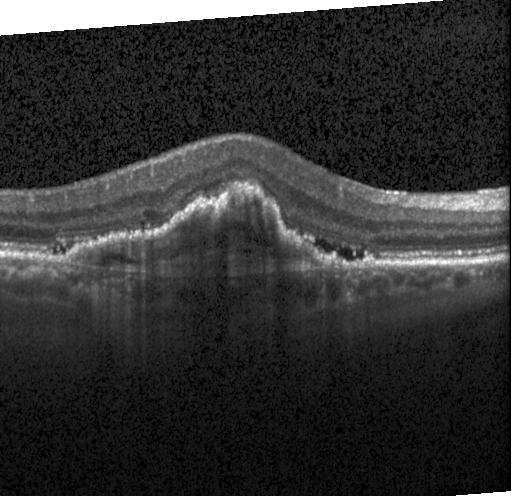
This B-scan demonstrates a choroidal neovascular membrane.